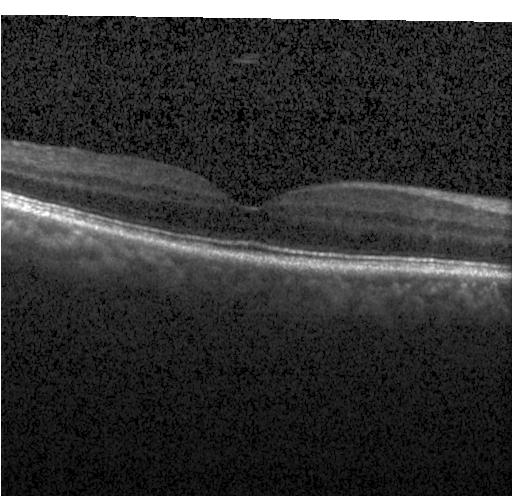
Dx: neither CNV, DME, nor drusen.